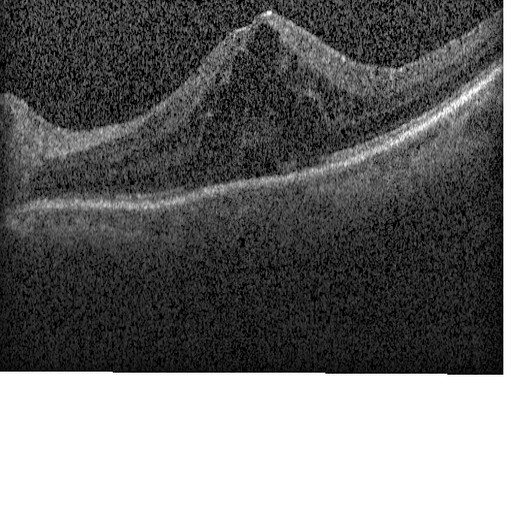 Spectral-domain optical coherence tomography · retinal OCT B-scan · acquired on a Heidelberg Spectralis · through the macula.
Diagnosis: diabetic macular edema (DME).